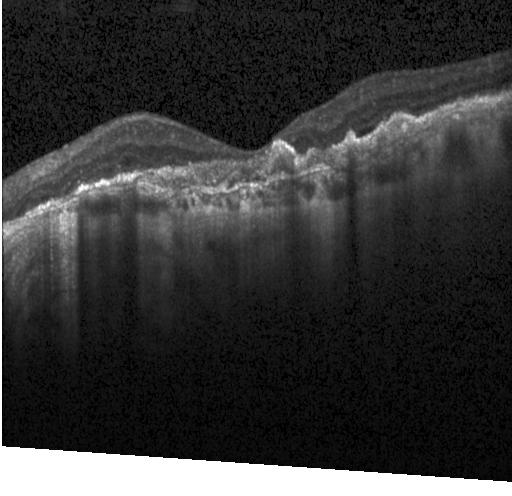 Assessment: choroidal neovascularization (CNV).